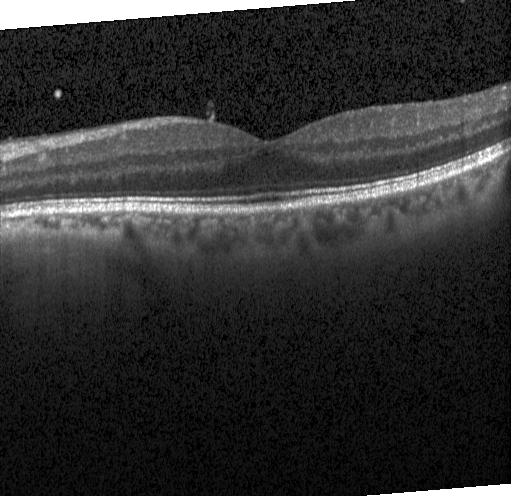
OCT scan showing no evidence of choroidal neovascularization, diabetic macular edema, or drusen.